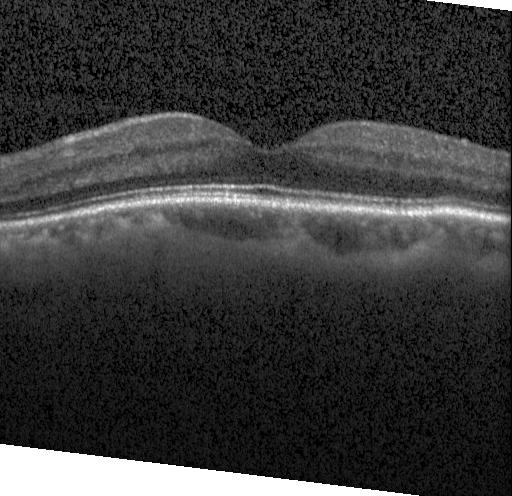

Assessment: no choroidal neovascularization, no diabetic macular edema, and no drusen.